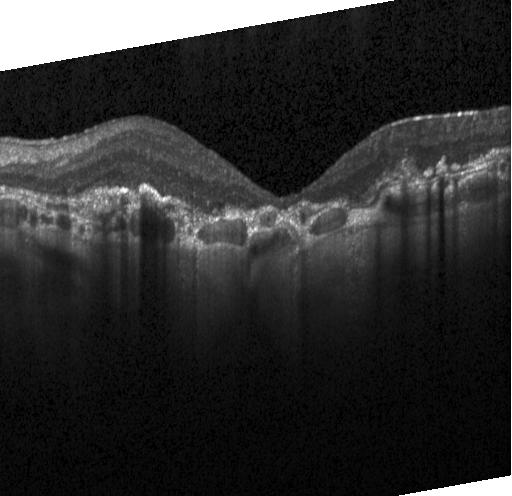
OCT scan showing choroidal neovascularization.